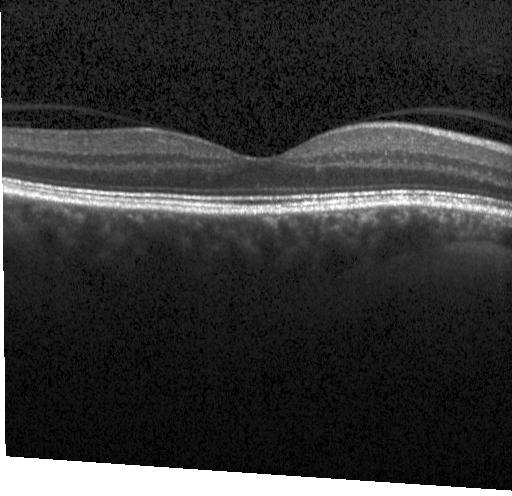 Optical coherence tomography scan. Instrument: Heidelberg Spectralis.
Finding: no choroidal neovascularization, no diabetic macular edema, and no drusen.